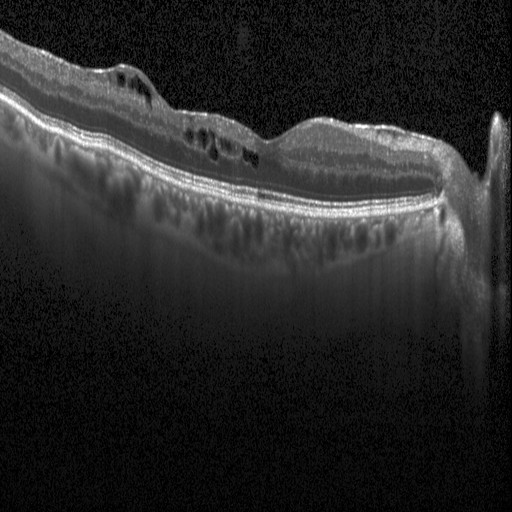 Through the macula; Heidelberg Spectralis OCT system; retinal OCT B-scan; SD-OCT
Finding: diabetic macular edema.